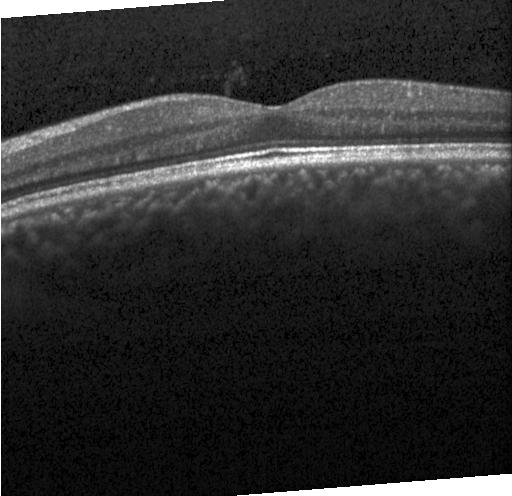

Retinal OCT cross-section. Diagnosis: neither CNV, DME, nor drusen.